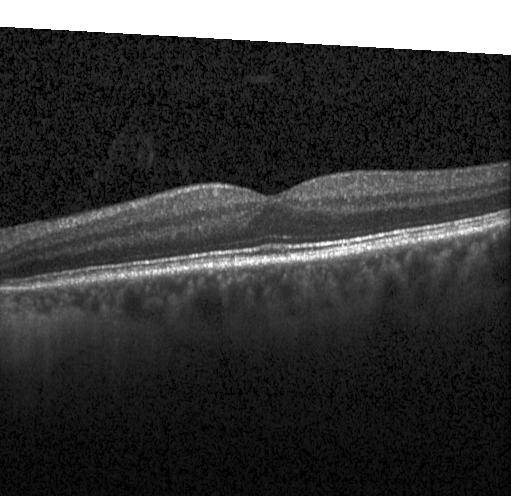
No evidence of choroidal neovascularization, diabetic macular edema, or drusen.